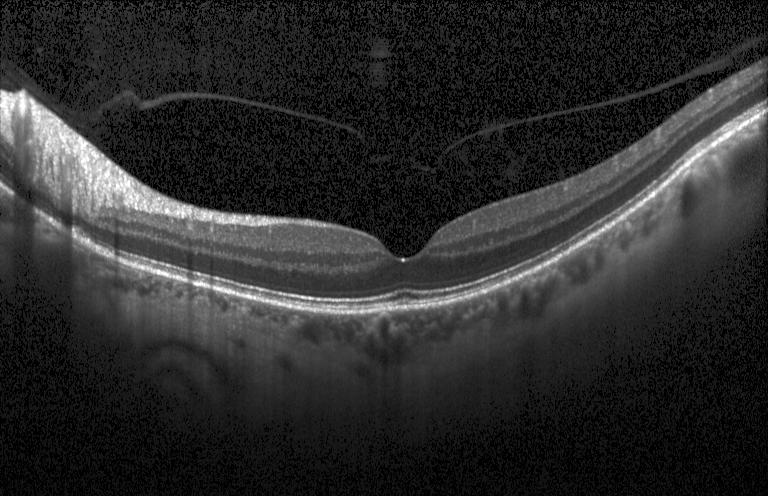
Dx: no CNV, DME, or drusen.